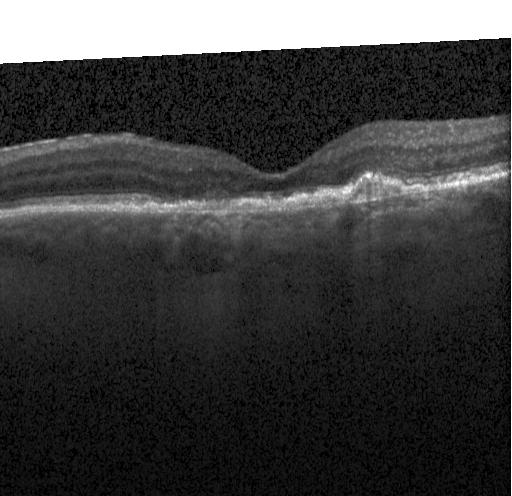

OCT scan showing choroidal neovascularization (CNV).